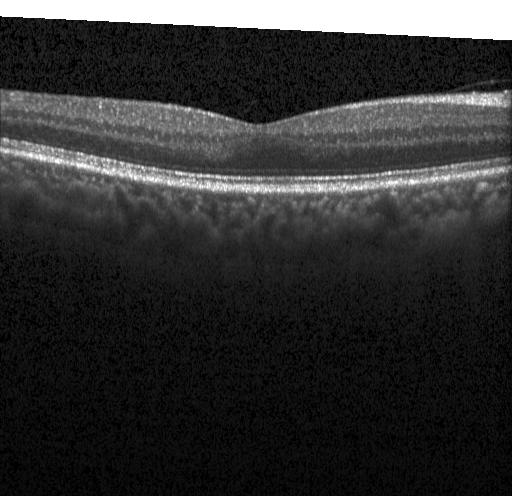

Horizontal scan through the fovea · retinal OCT B-scan · SD-OCT — This B-scan demonstrates neither CNV, DME, nor drusen.